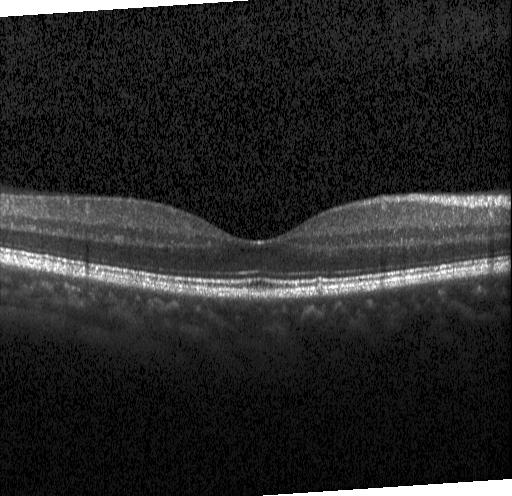
Optical coherence tomography B-scan. Spectral-domain OCT. Assessment: neither choroidal neovascularization, diabetic macular edema, nor drusen.